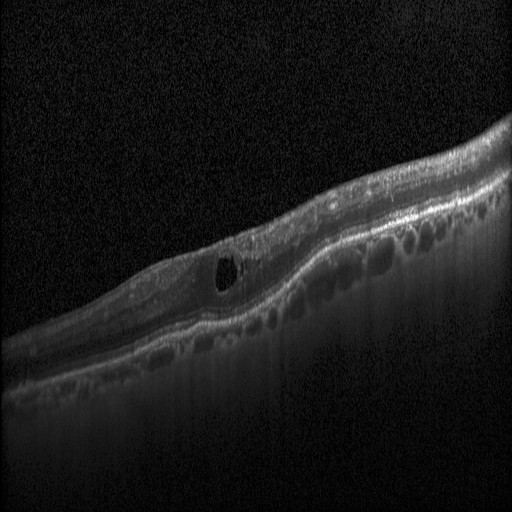 Fovea-centered, instrument: Heidelberg Spectralis, optical coherence tomography scan, SD-OCT
OCT finding: diabetic macular edema (DME).